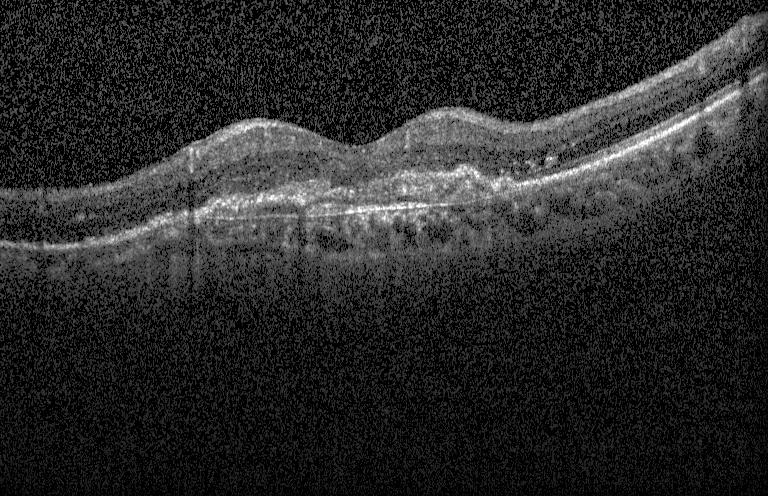
Macular OCT: a choroidal neovascular membrane.